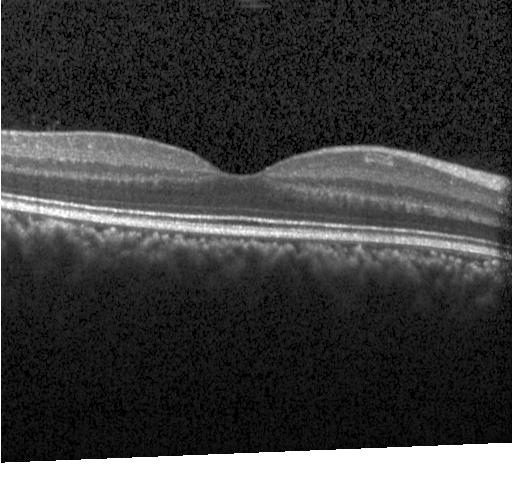 Retinal OCT cross-section.
Dx: neither choroidal neovascularization, diabetic macular edema, nor drusen.